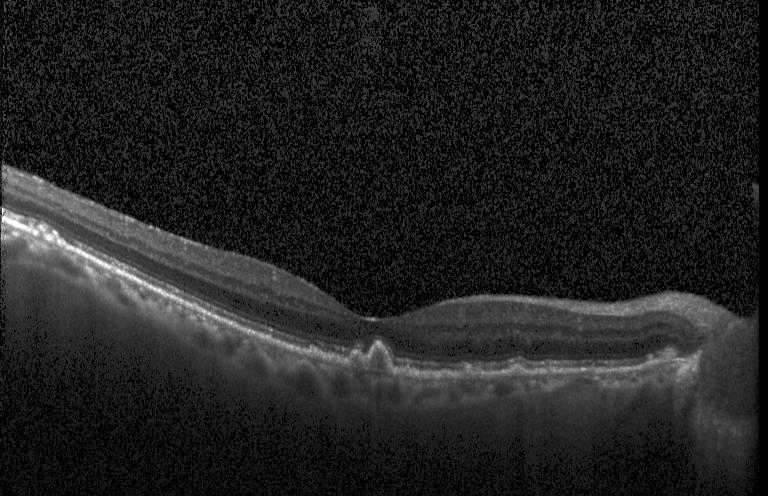 Dx: drusen.